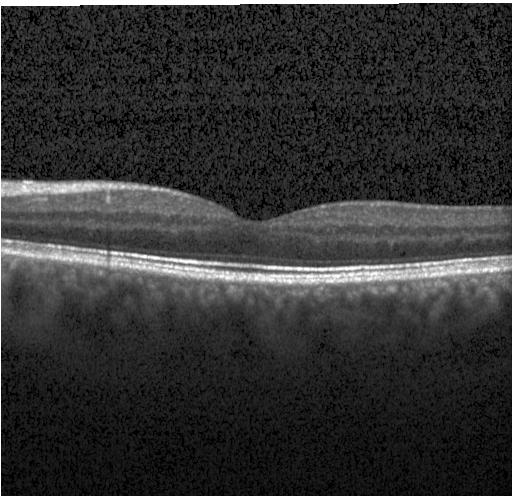 OCT B-scan
Finding: no evidence of CNV, DME, or drusen.